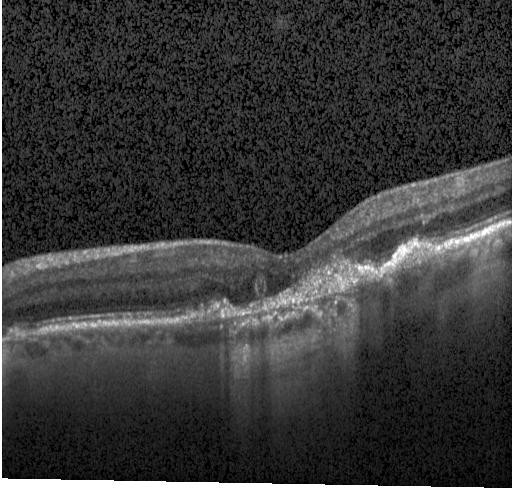 Retinal OCT cross-section. Spectral-domain OCT
Finding: choroidal neovascularization.